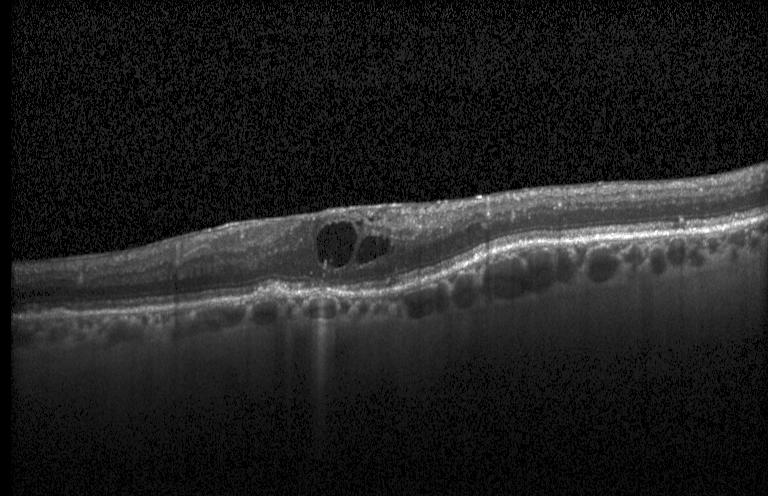
Diagnosis: choroidal neovascularization (CNV).